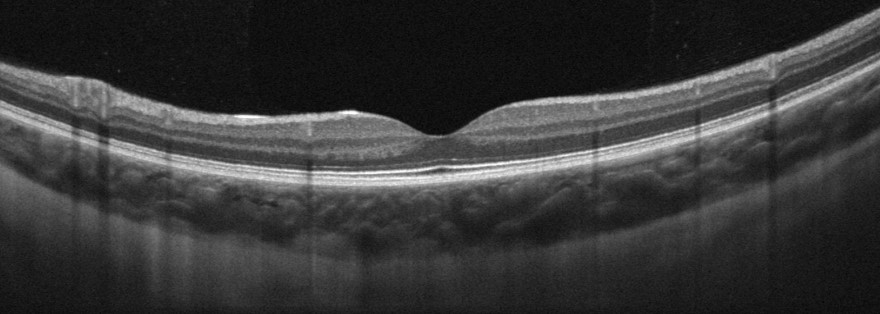

Retinal OCT B-scan; acquired on an Optovue Avanti RTVue XR; fovea-centered.
Diagnosis: no AMD, DME, ERM, RAO, RVO, or VID.